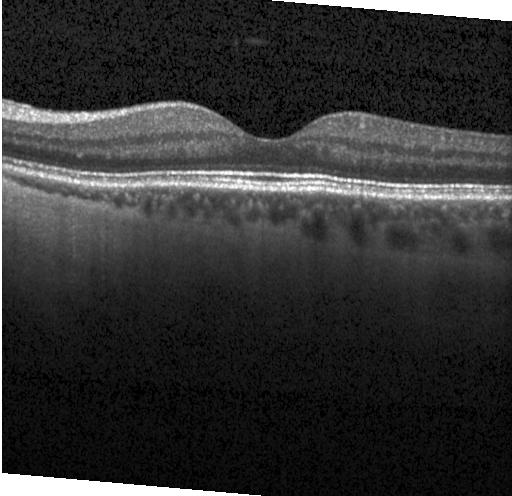 Dx: neither choroidal neovascularization, diabetic macular edema, nor drusen.